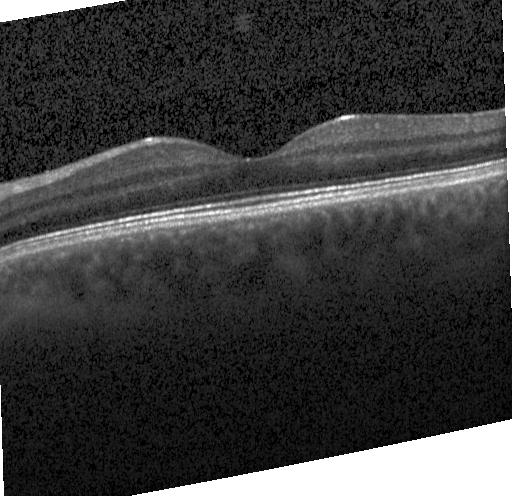
Retinal OCT B-scan. Instrument: Heidelberg Spectralis. Spectral-domain optical coherence tomography. Horizontal scan through the fovea
Finding: no choroidal neovascularization, no diabetic macular edema, and no drusen.